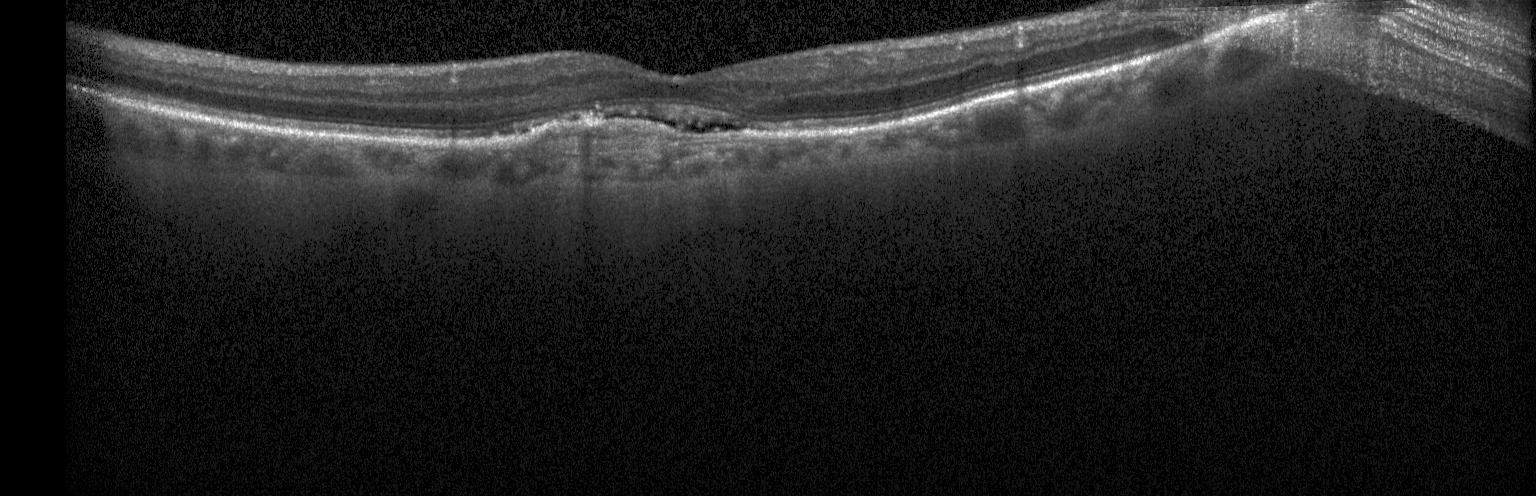

Optical coherence tomography B-scan. This B-scan demonstrates CNV.